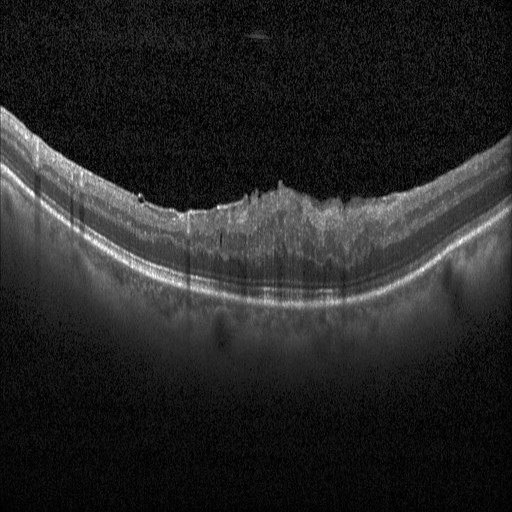
OCT B-scan. Macular OCT: DME.